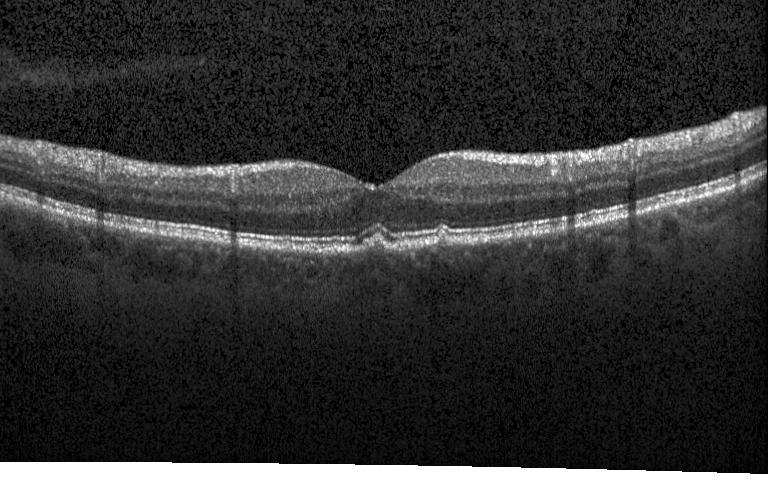

Impression: sub-RPE drusenoid deposits.